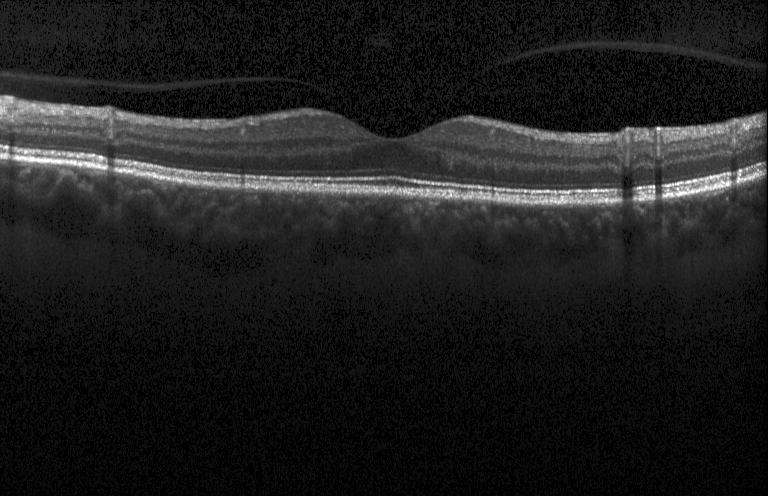 Through the macula. Acquired on a Heidelberg Spectralis. OCT B-scan — Macular OCT: neither choroidal neovascularization, diabetic macular edema, nor drusen.